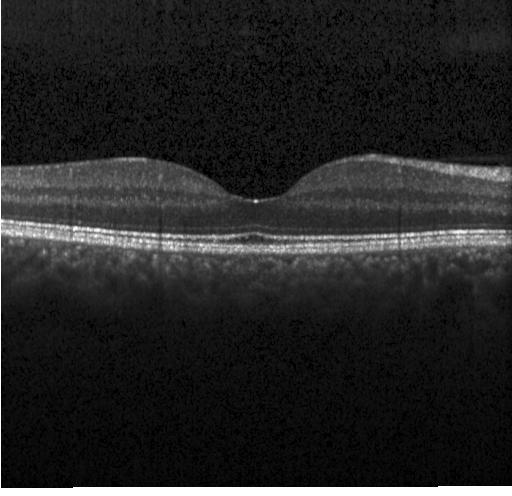

This B-scan demonstrates no choroidal neovascularization, no diabetic macular edema, and no drusen.